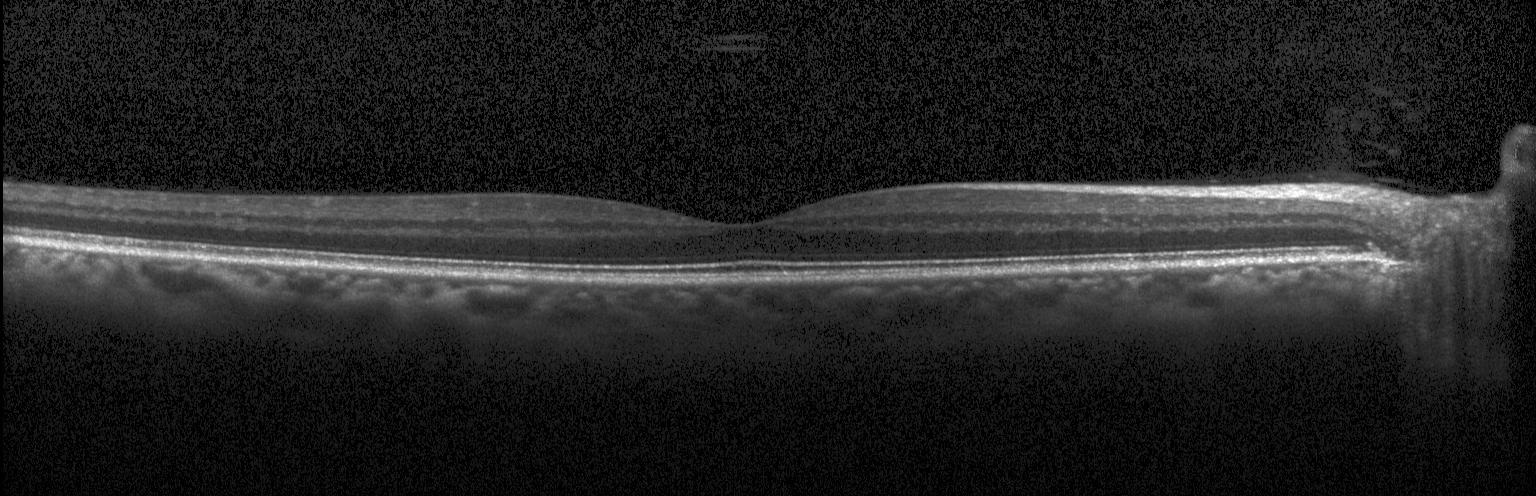
Impression: neither CNV, DME, nor drusen.